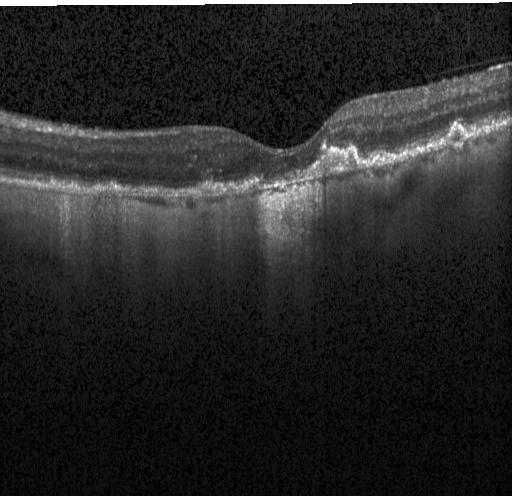 OCT line scan. Through the macula. This B-scan demonstrates choroidal neovascularization.